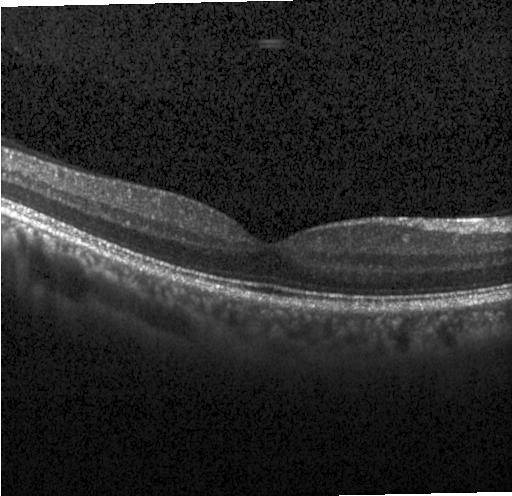 Instrument: Heidelberg Spectralis; OCT line scan; horizontal scan through the fovea. OCT finding: neither CNV, DME, nor drusen.